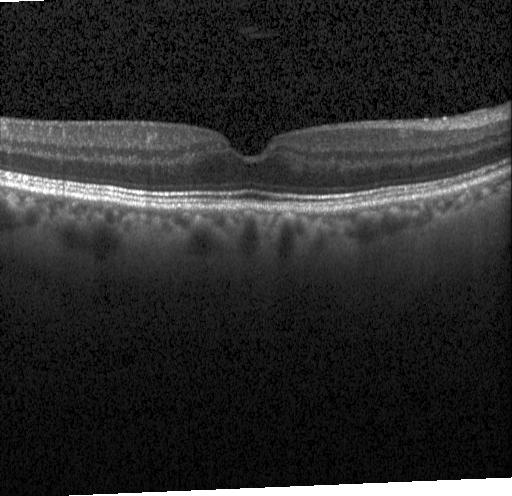 OCT line scan.
Diagnosis: neither choroidal neovascularization, diabetic macular edema, nor drusen.